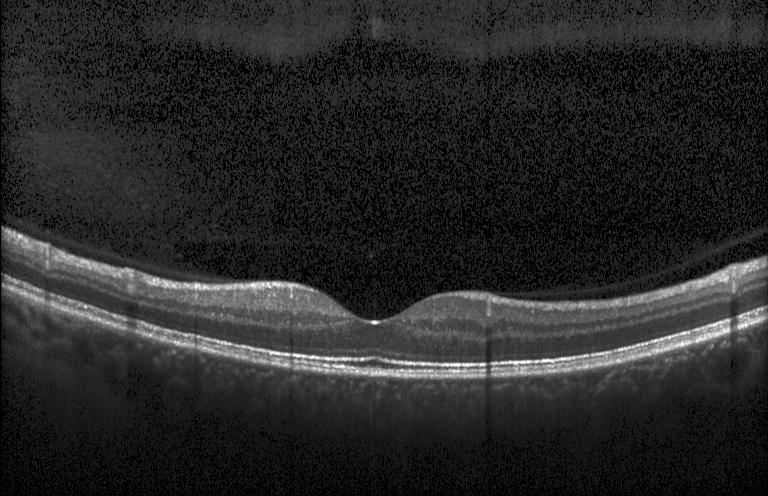

Diagnosis: no CNV, DME, or drusen.